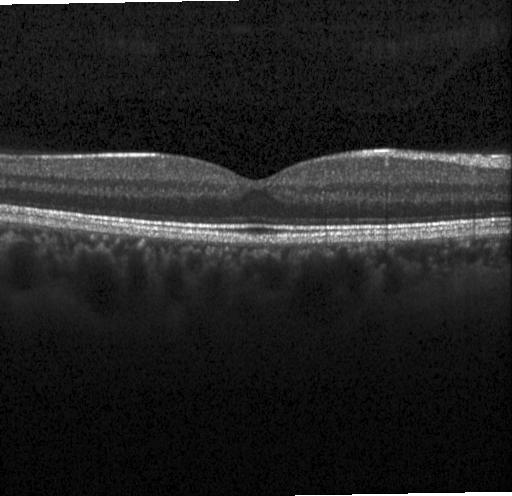
OCT finding: no choroidal neovascularization, diabetic macular edema, or drusen.